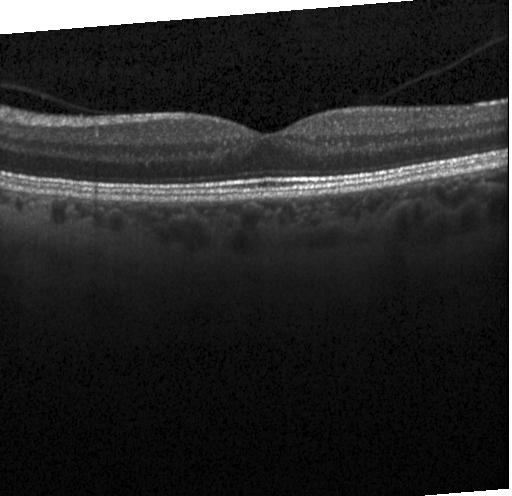 Optical coherence tomography scan
No evidence of CNV, DME, or drusen.